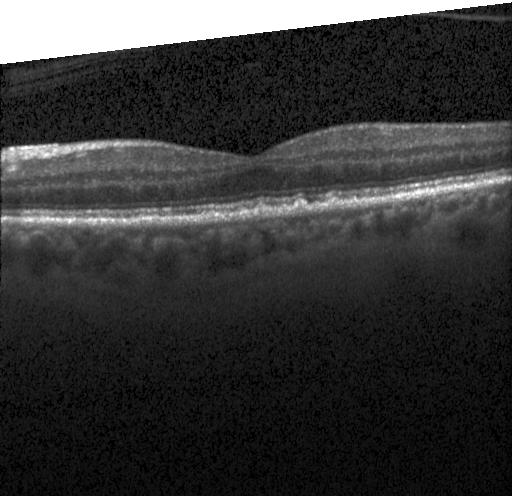 Multiple drusen.